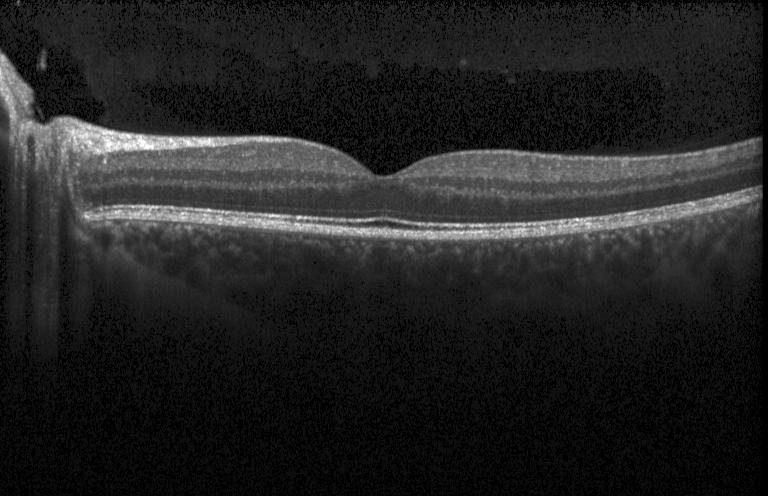 OCT B-scan — Finding: neither choroidal neovascularization, diabetic macular edema, nor drusen.